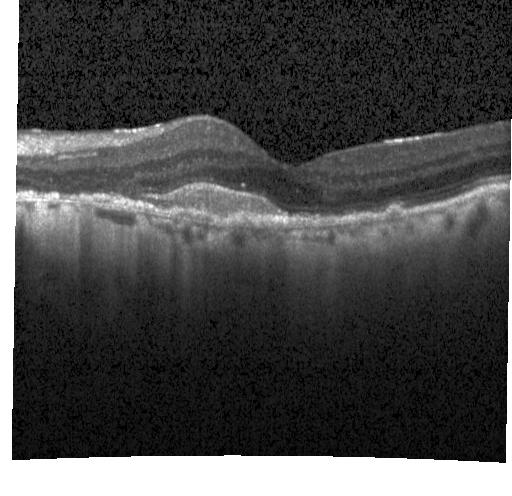 OCT line scan.
Finding: choroidal neovascularization.